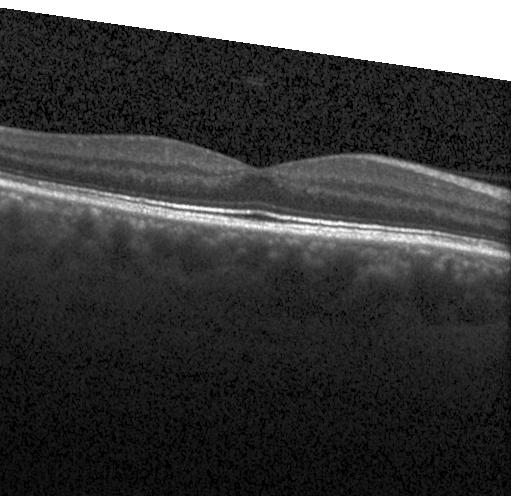

Dx: no CNV, DME, or drusen.